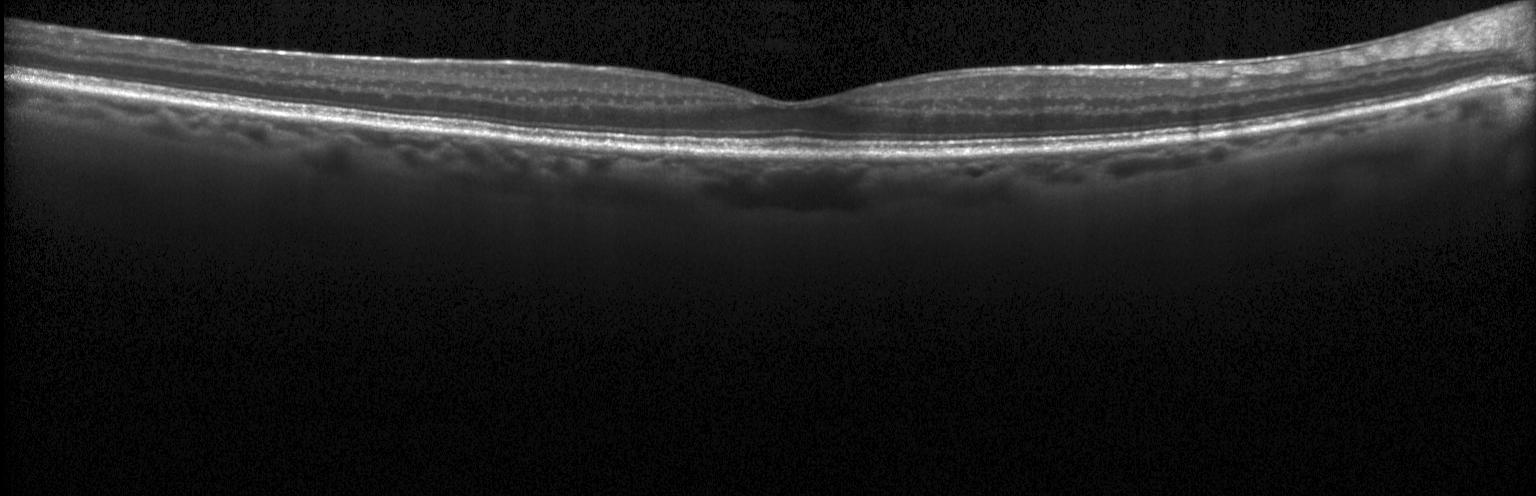 Neither choroidal neovascularization, diabetic macular edema, nor drusen.